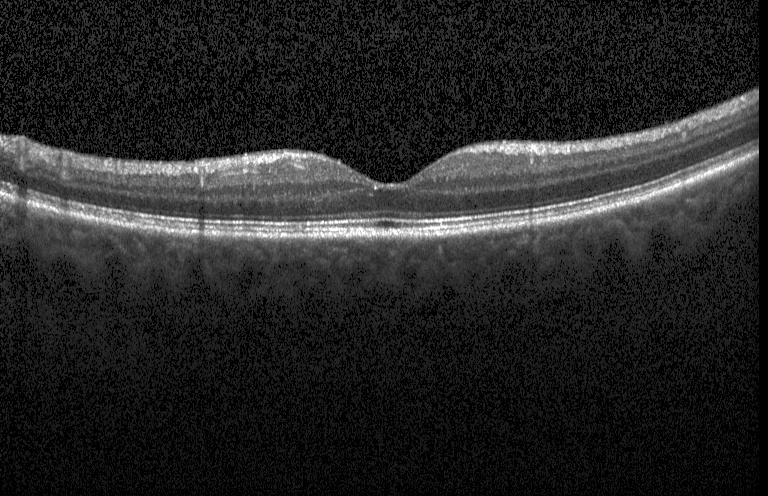 Retinal OCT cross-section — Diagnosis: no evidence of choroidal neovascularization, diabetic macular edema, or drusen.